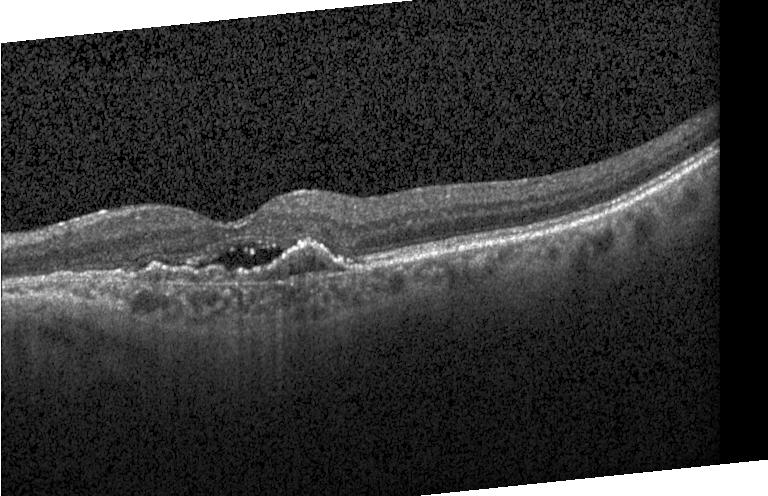
Retinal OCT B-scan — This B-scan demonstrates a choroidal neovascular membrane.